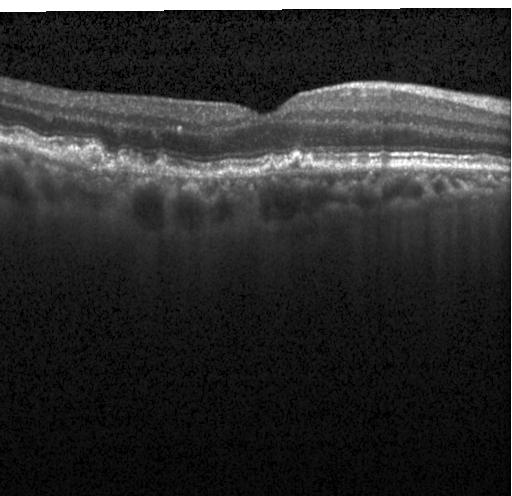
Instrument: Heidelberg Spectralis; through the macula; spectral-domain OCT; retinal OCT B-scan. Assessment: multiple drusen.